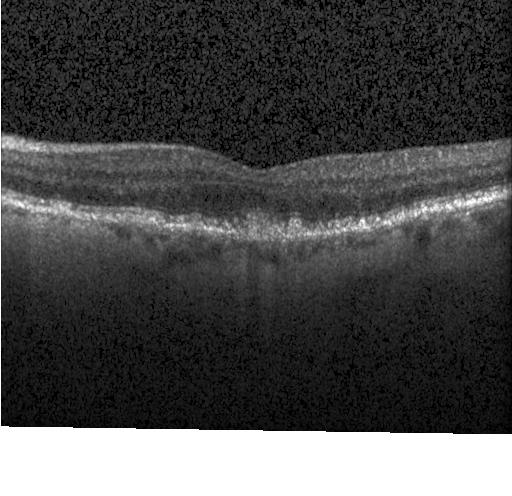

Impression: drusen.